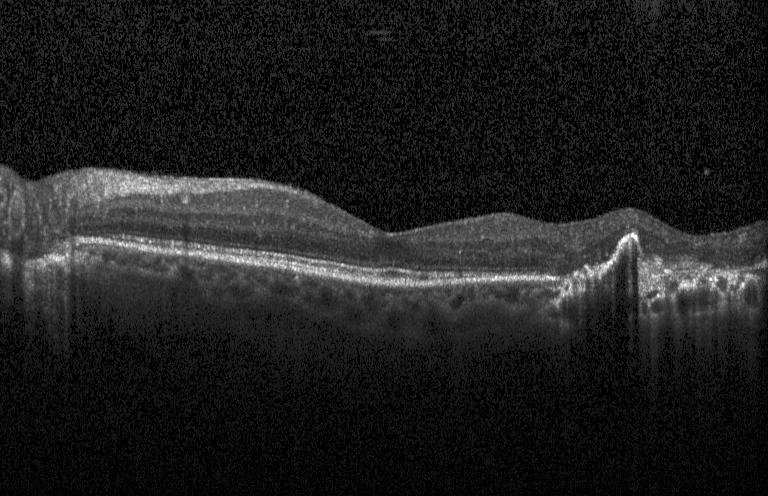
Impression: choroidal neovascularization (CNV).